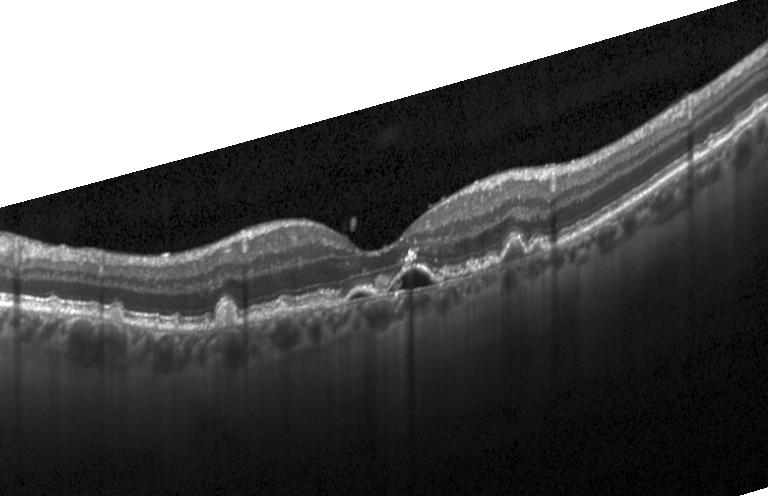
Macular OCT demonstrating a choroidal neovascular membrane.